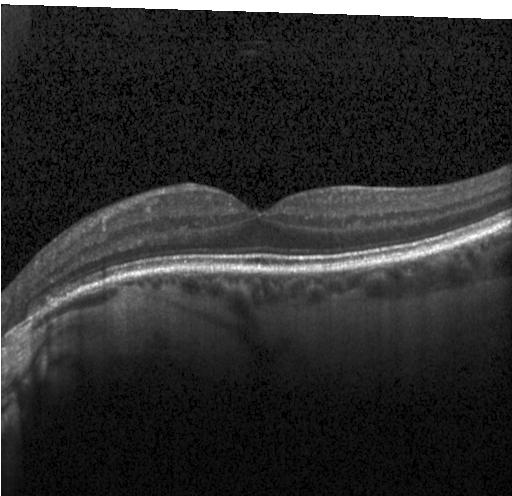

OCT finding: no CNV, no DME, and no drusen.